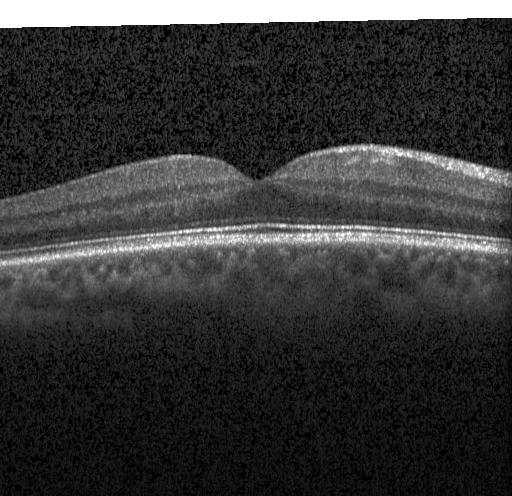

Dx: no evidence of choroidal neovascularization, diabetic macular edema, or drusen.